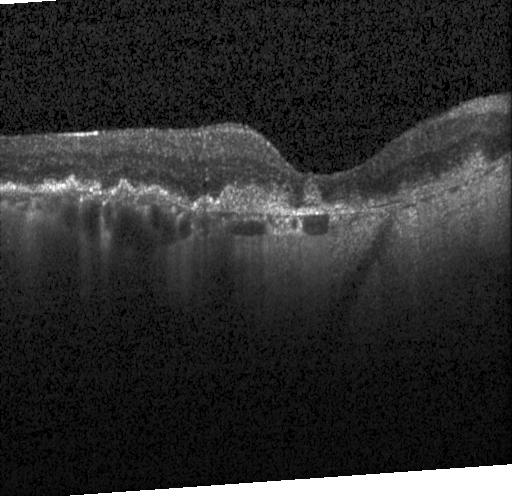

Optical coherence tomography B-scan — Diagnosis: a choroidal neovascular membrane.